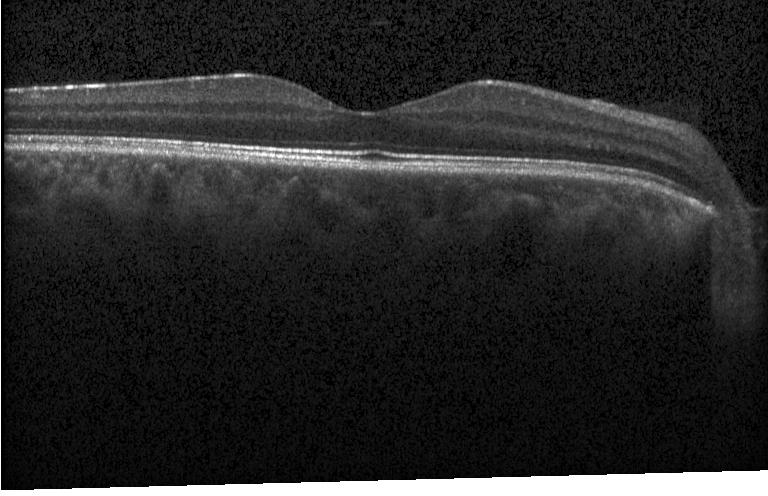
Macular OCT: no evidence of choroidal neovascularization, diabetic macular edema, or drusen.